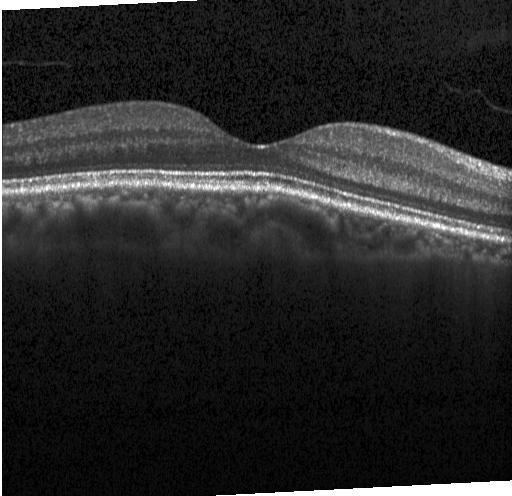
Spectral-domain OCT B-scan: no evidence of CNV, DME, or drusen.